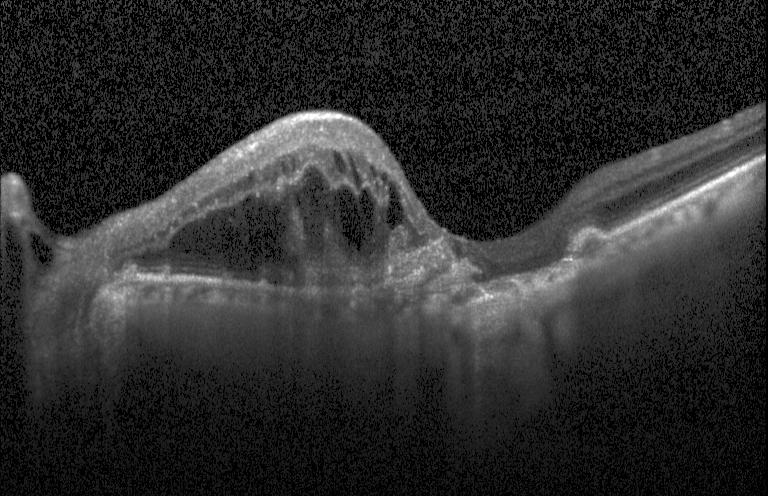

Through the macula; spectral-domain OCT; retinal OCT cross-section.
Diagnosis: a choroidal neovascular membrane.